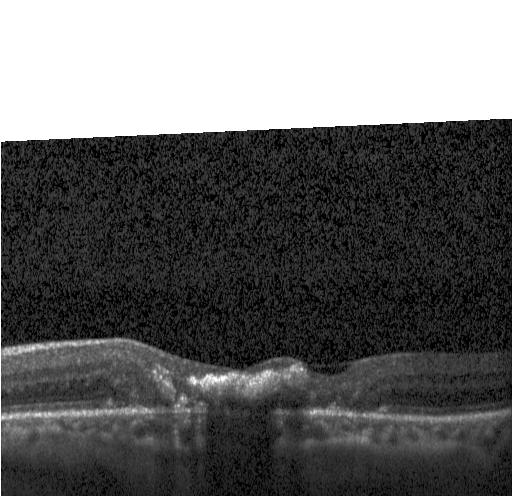
Spectral-domain optical coherence tomography. OCT line scan. Heidelberg Spectralis OCT system. Horizontal scan through the fovea
Macular OCT: a choroidal neovascular membrane.